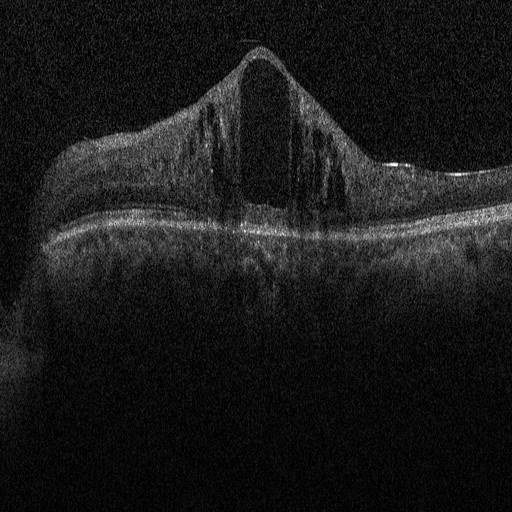 Acquired on a Heidelberg Spectralis. Retinal OCT cross-section. Diagnosis: DME.